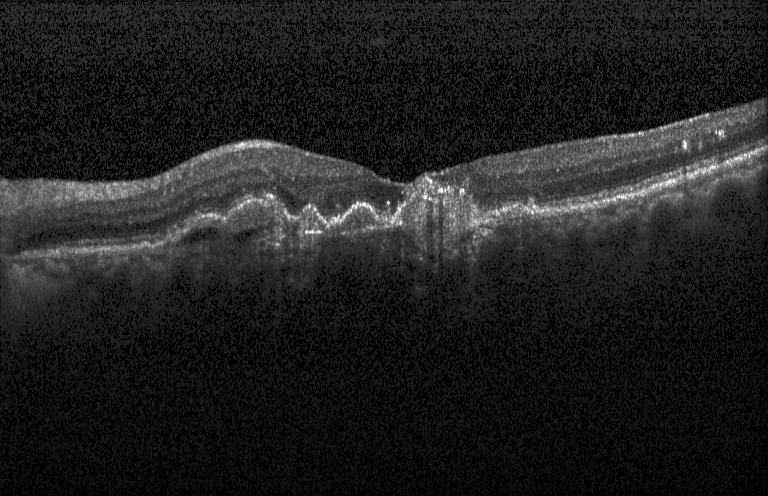

Optical coherence tomography B-scan — Dx: a choroidal neovascular membrane.